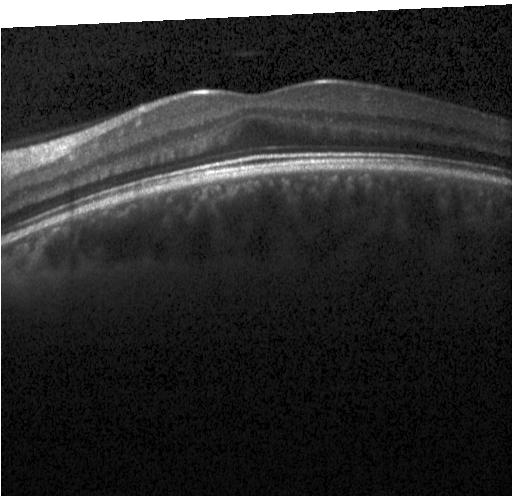
OCT B-scan.
Neither choroidal neovascularization, diabetic macular edema, nor drusen.